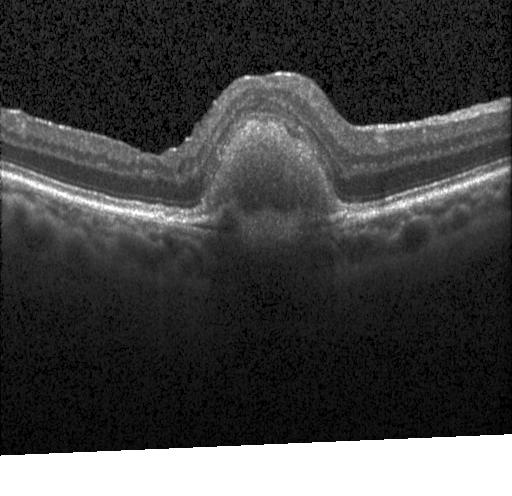

Retinal OCT cross-section
Finding: a choroidal neovascular membrane.